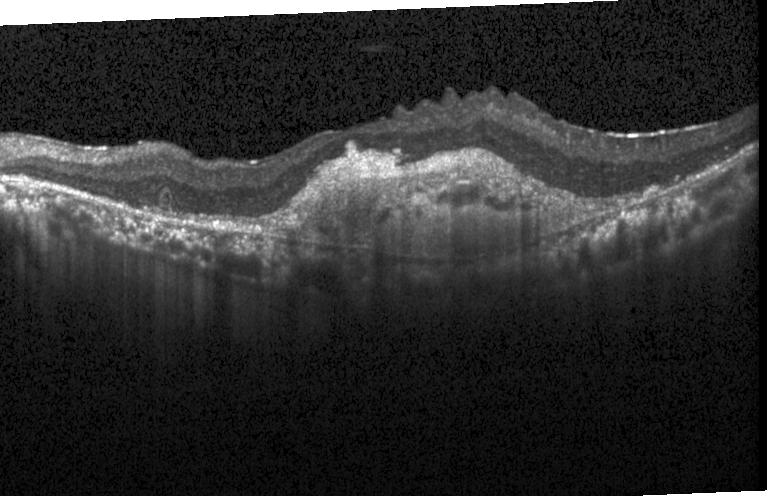

Optical coherence tomography B-scan. Diagnosis: a choroidal neovascular membrane.